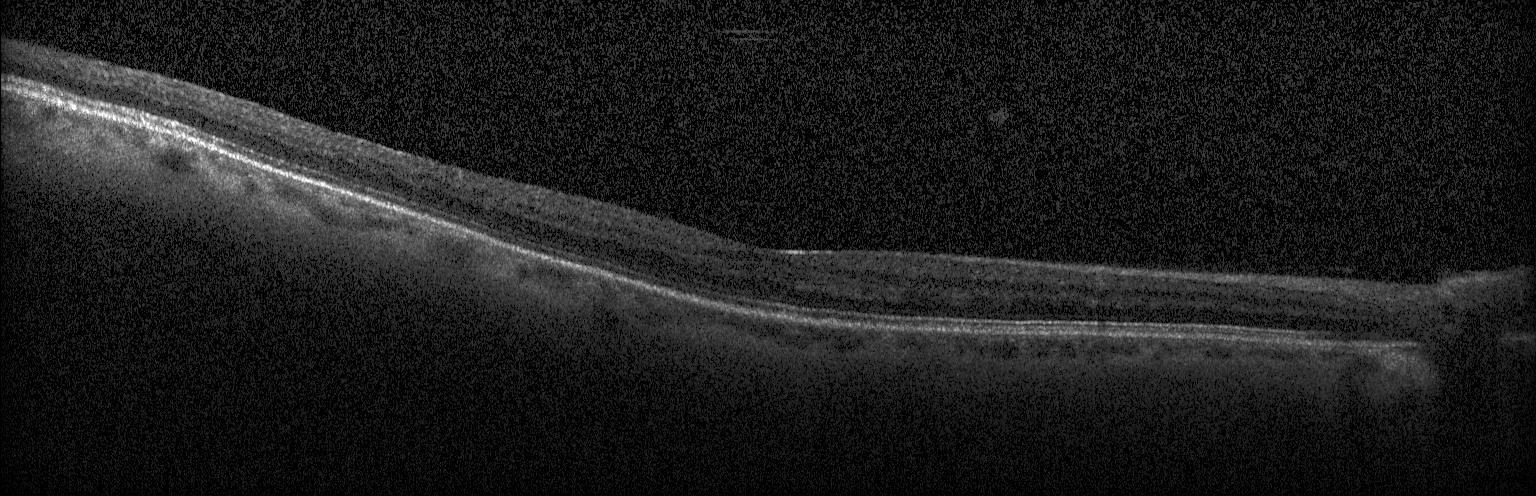

Optical coherence tomography B-scan, SD-OCT. OCT finding: no choroidal neovascularization, no diabetic macular edema, and no drusen.